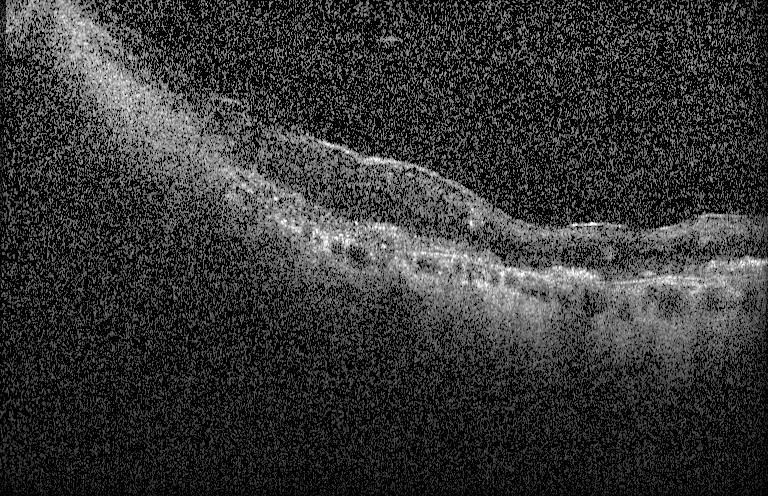

Spectral-domain optical coherence tomography · optical coherence tomography scan · Heidelberg Spectralis.
Assessment: CNV.